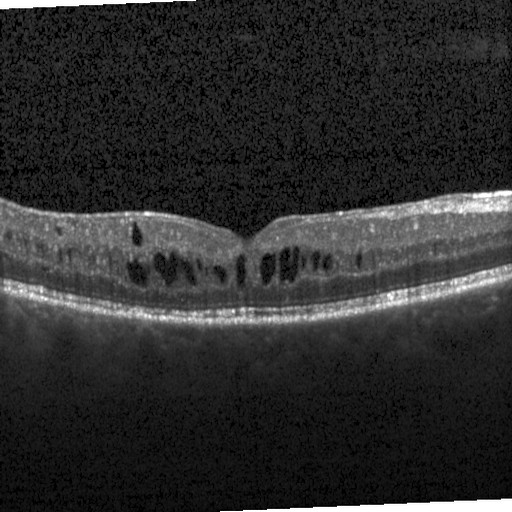
Macular OCT: diabetic macular edema.